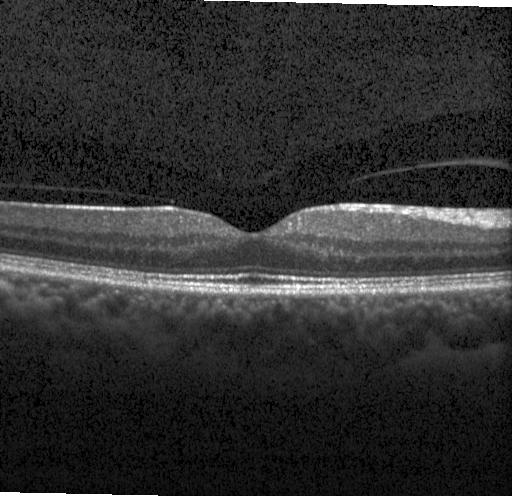 OCT B-scan showing no evidence of choroidal neovascularization, diabetic macular edema, or drusen.